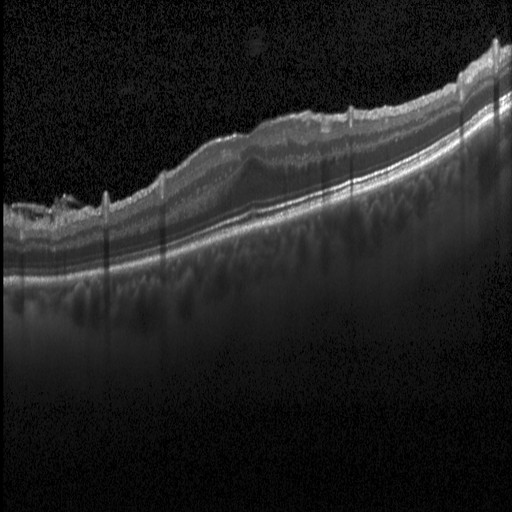 Centered on the fovea; OCT B-scan; SD-OCT; acquired on a Heidelberg Spectralis.
Diabetic macular edema.